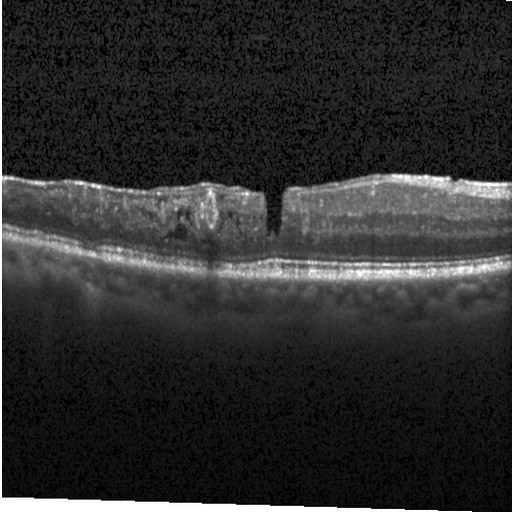 Dx: diabetic macular edema (DME).